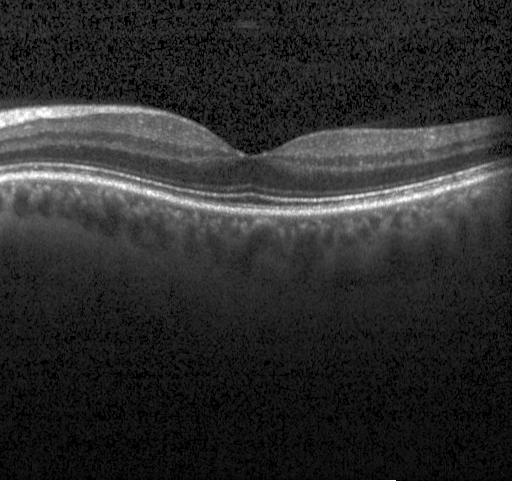
Optical coherence tomography B-scan.
Diagnosis: no evidence of choroidal neovascularization, diabetic macular edema, or drusen.